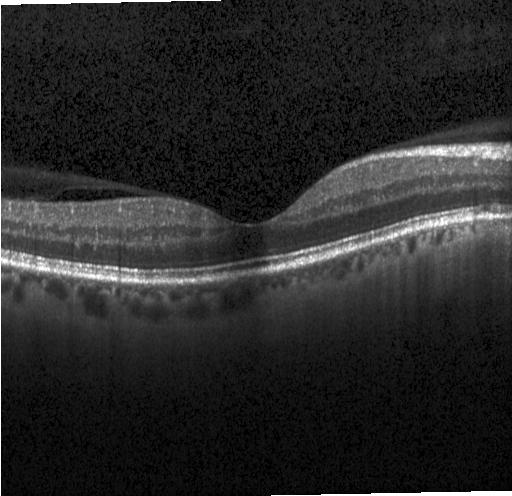 Retinal OCT B-scan, centered on the fovea.
Macular OCT: neither CNV, DME, nor drusen.